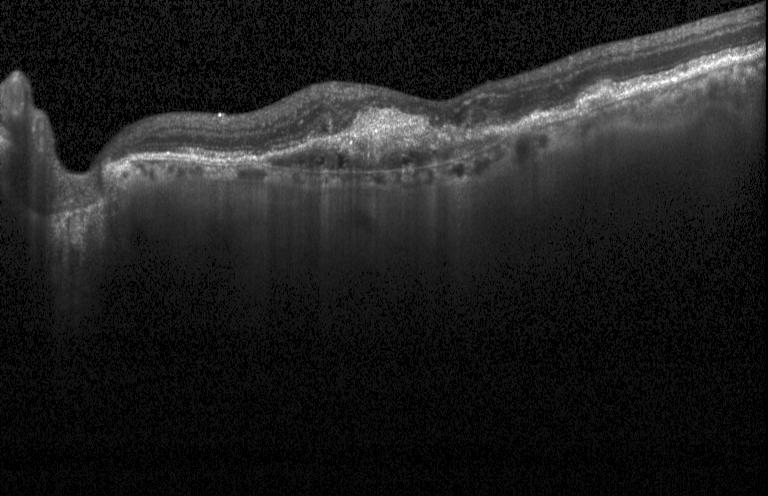

Retinal OCT cross-section.
This B-scan demonstrates choroidal neovascularization (CNV).